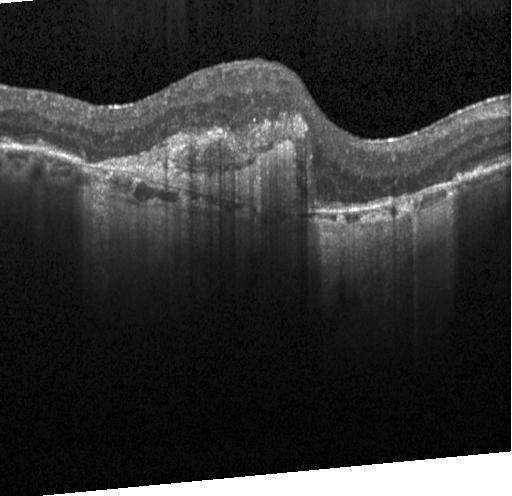 Retinal OCT B-scan
Macular OCT: a choroidal neovascular membrane.